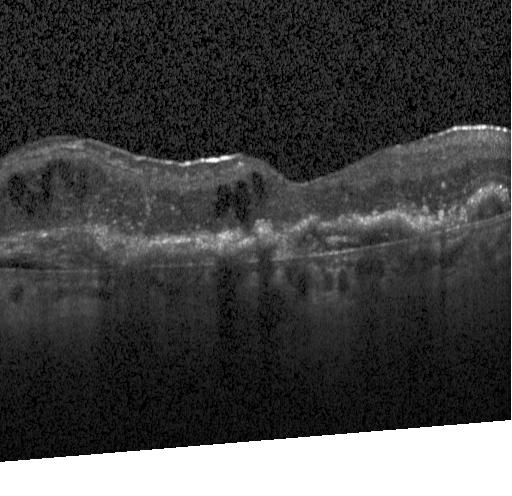

Optical coherence tomography scan. Heidelberg Spectralis. Spectral-domain OCT
A choroidal neovascular membrane.